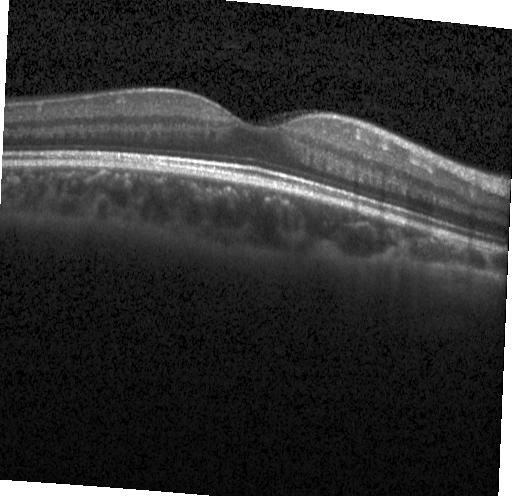

OCT finding: no choroidal neovascularization, no diabetic macular edema, and no drusen.